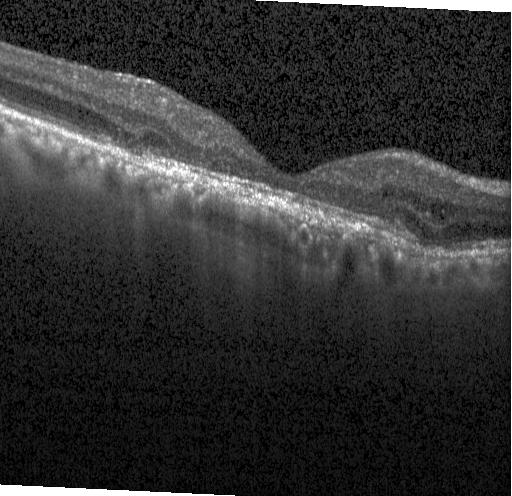 OCT line scan · Heidelberg Spectralis.
Assessment: choroidal neovascularization.